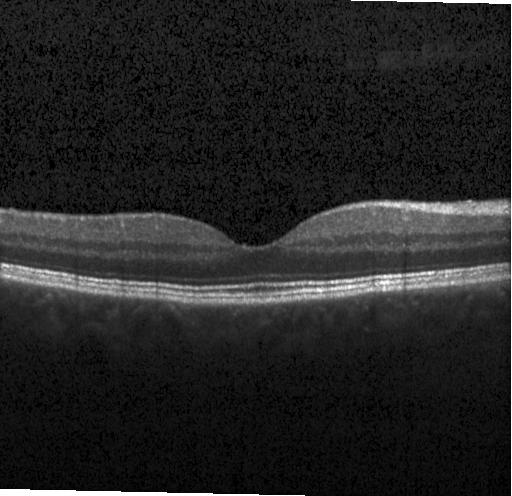 Retinal OCT cross-section showing neither CNV, DME, nor drusen.